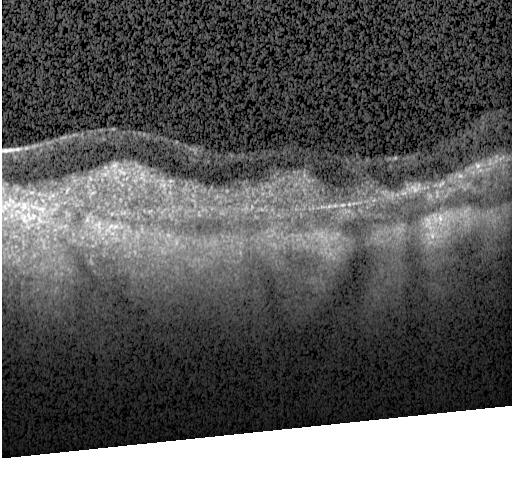
Retinal OCT B-scan · centered on the fovea · SD-OCT · Heidelberg Spectralis — Macular OCT: a choroidal neovascular membrane.